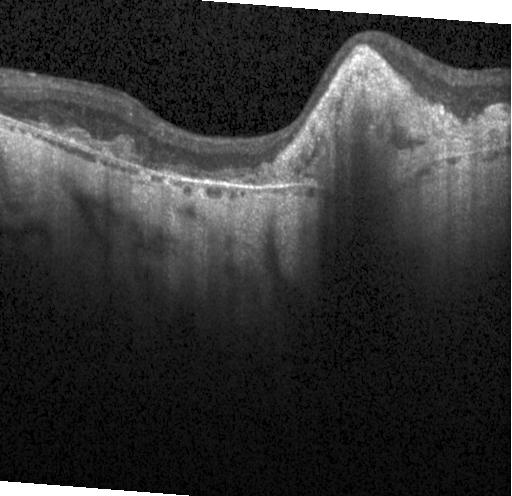
Macular scan, retinal OCT B-scan, SD-OCT — Finding: choroidal neovascularization.